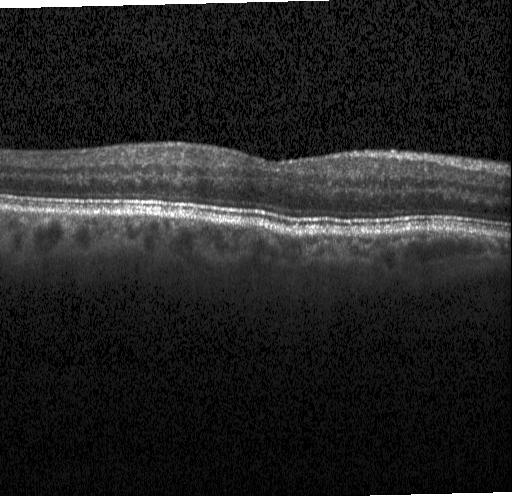 Retinal OCT B-scan.
Macular OCT: no choroidal neovascularization, diabetic macular edema, or drusen.